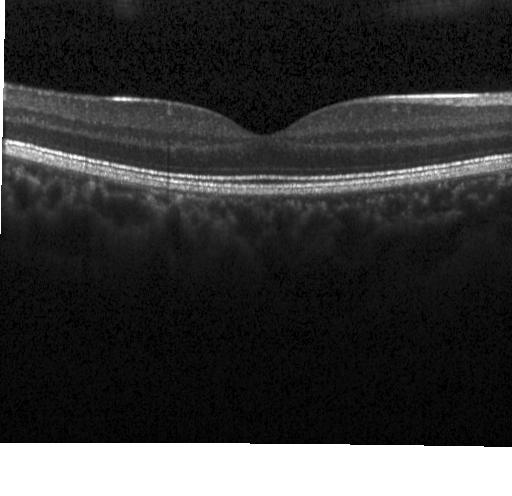

OCT line scan
This B-scan demonstrates neither choroidal neovascularization, diabetic macular edema, nor drusen.